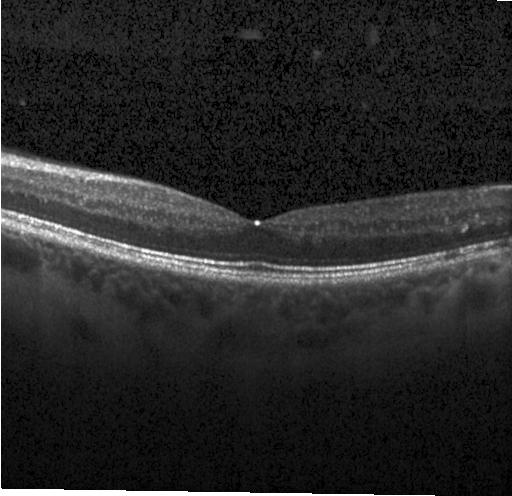
Instrument: Heidelberg Spectralis; optical coherence tomography scan; spectral-domain OCT.
Diagnosis: no CNV, DME, or drusen.